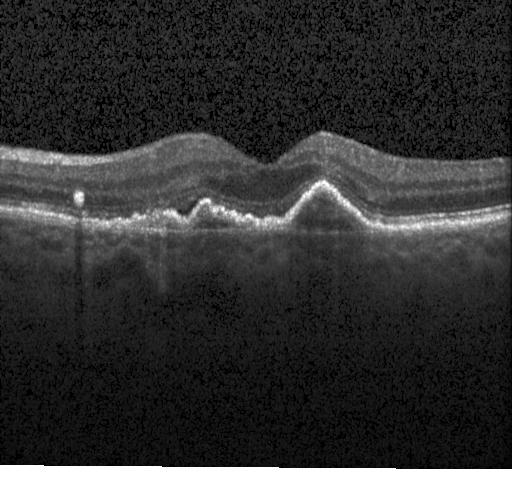

Optical coherence tomography scan · Heidelberg Spectralis OCT system.
Impression: choroidal neovascularization (CNV).